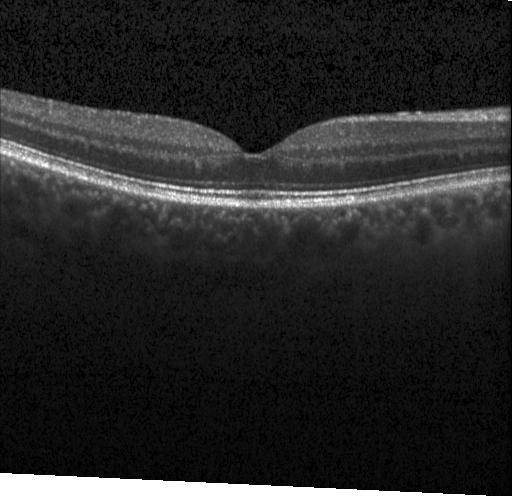

Centered on the fovea; spectral-domain optical coherence tomography; instrument: Heidelberg Spectralis; OCT B-scan. Finding: no evidence of choroidal neovascularization, diabetic macular edema, or drusen.